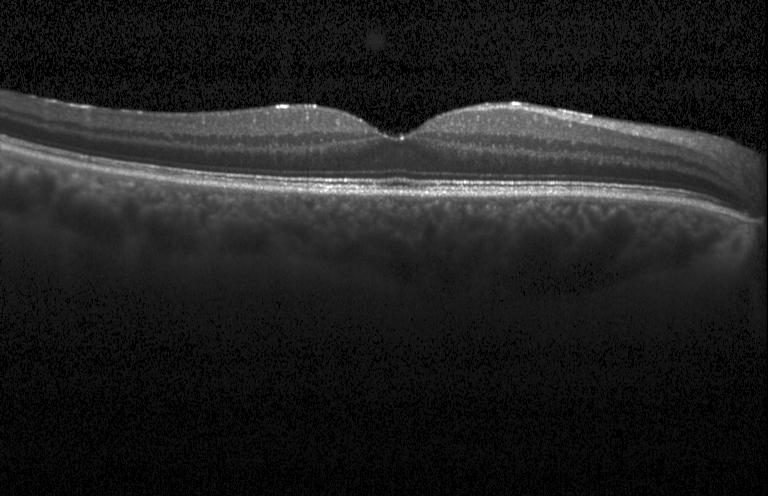
OCT B-scan showing no choroidal neovascularization, diabetic macular edema, or drusen.